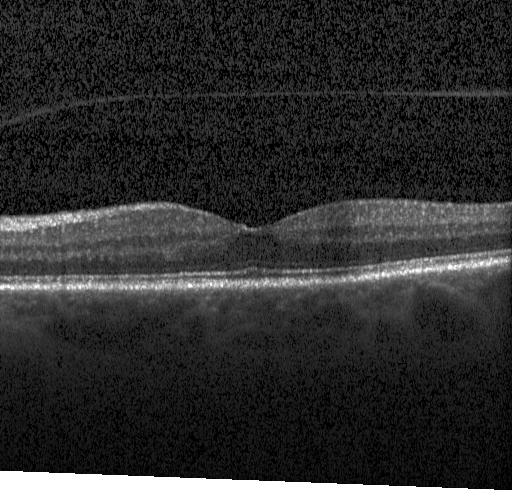

OCT finding: no choroidal neovascularization, diabetic macular edema, or drusen.